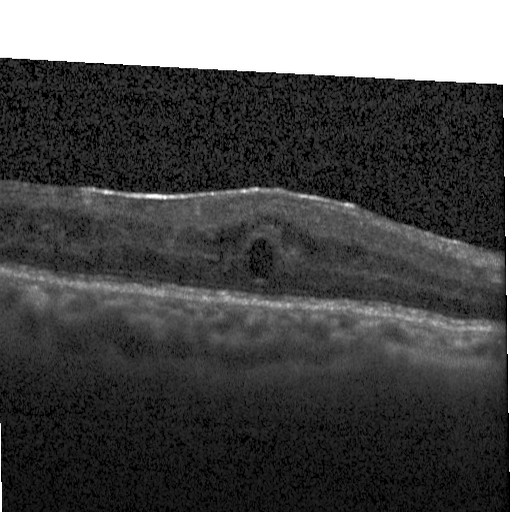 Optical coherence tomography B-scan. Spectral-domain OCT. Finding: diabetic macular edema (DME).